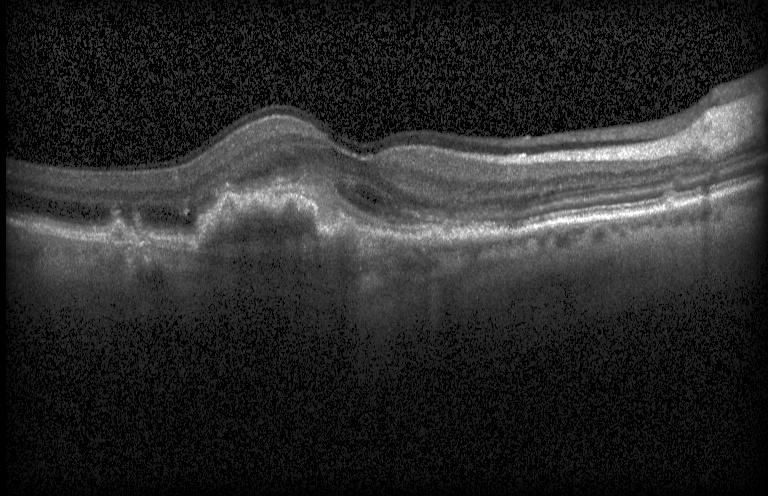

Macular OCT: a choroidal neovascular membrane.